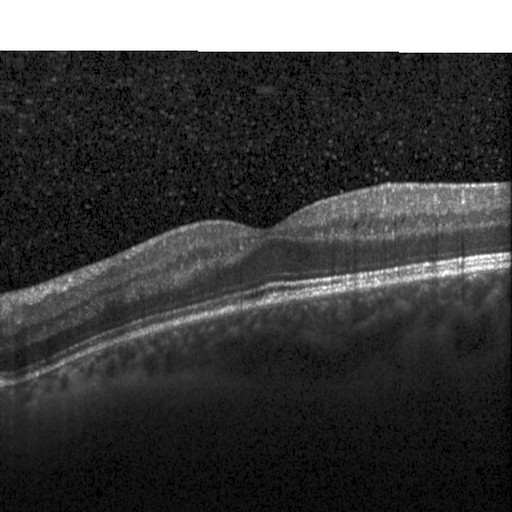
Heidelberg Spectralis, horizontal scan through the fovea, OCT B-scan — Impression: diabetic macular edema.